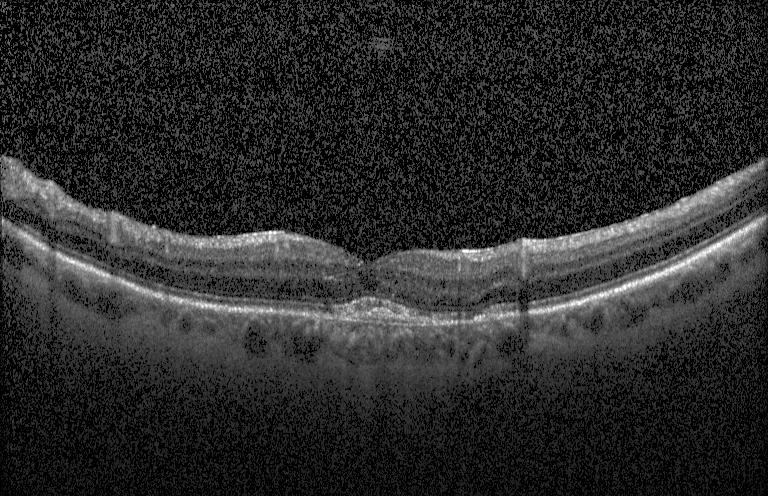
Finding: CNV.